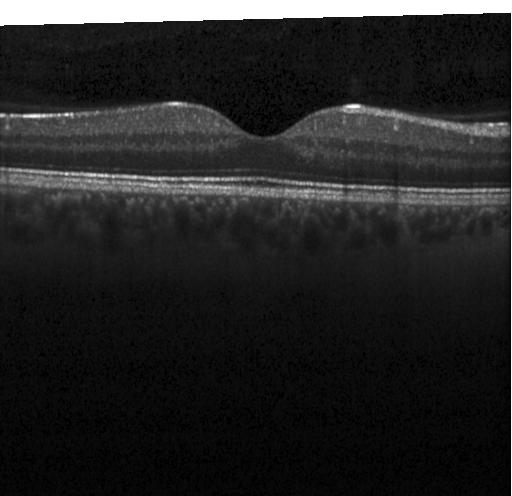
Spectral-domain OCT, macular scan, Heidelberg Spectralis OCT system, optical coherence tomography B-scan. This B-scan demonstrates no evidence of choroidal neovascularization, diabetic macular edema, or drusen.